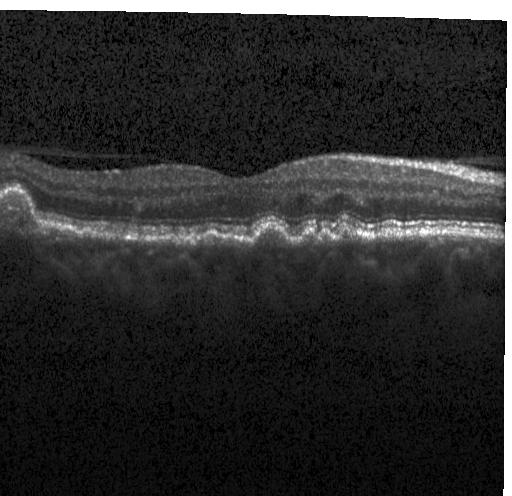

Heidelberg Spectralis. Centered on the fovea. Retinal OCT cross-section. Spectral-domain OCT. Impression: multiple drusen.